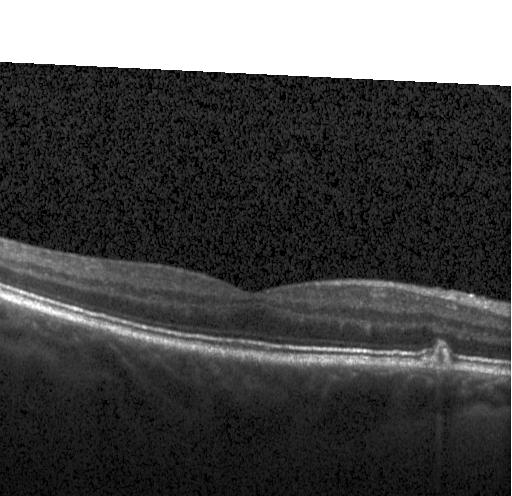

Centered on the fovea · optical coherence tomography scan · spectral-domain optical coherence tomography · instrument: Heidelberg Spectralis
Assessment: multiple drusen.